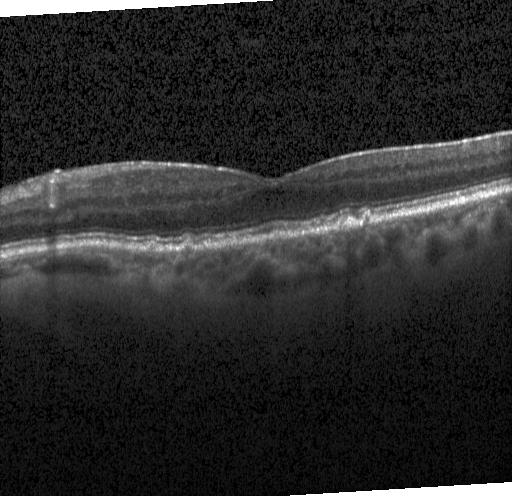
Finding: sub-RPE drusenoid deposits.